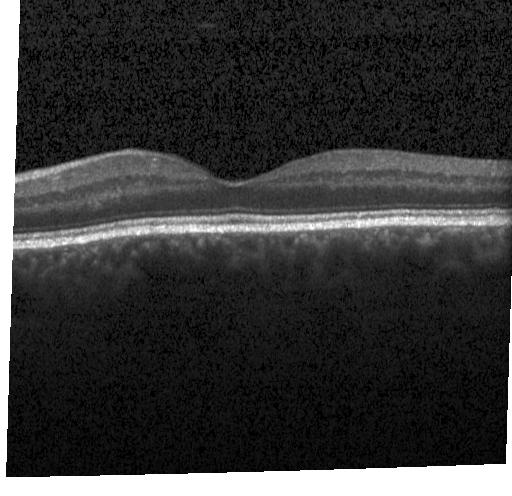 Spectral-domain OCT B-scan: no evidence of CNV, DME, or drusen.